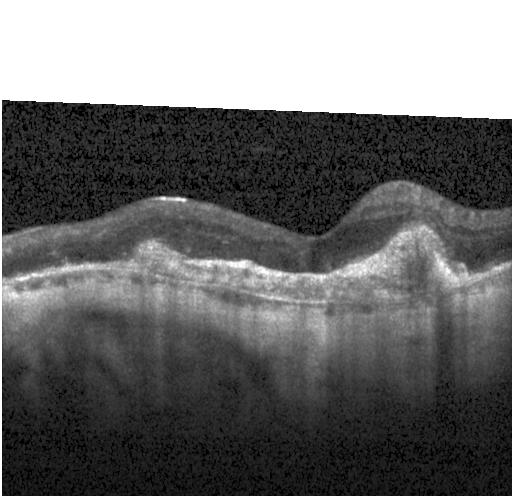

The scan shows a choroidal neovascular membrane.